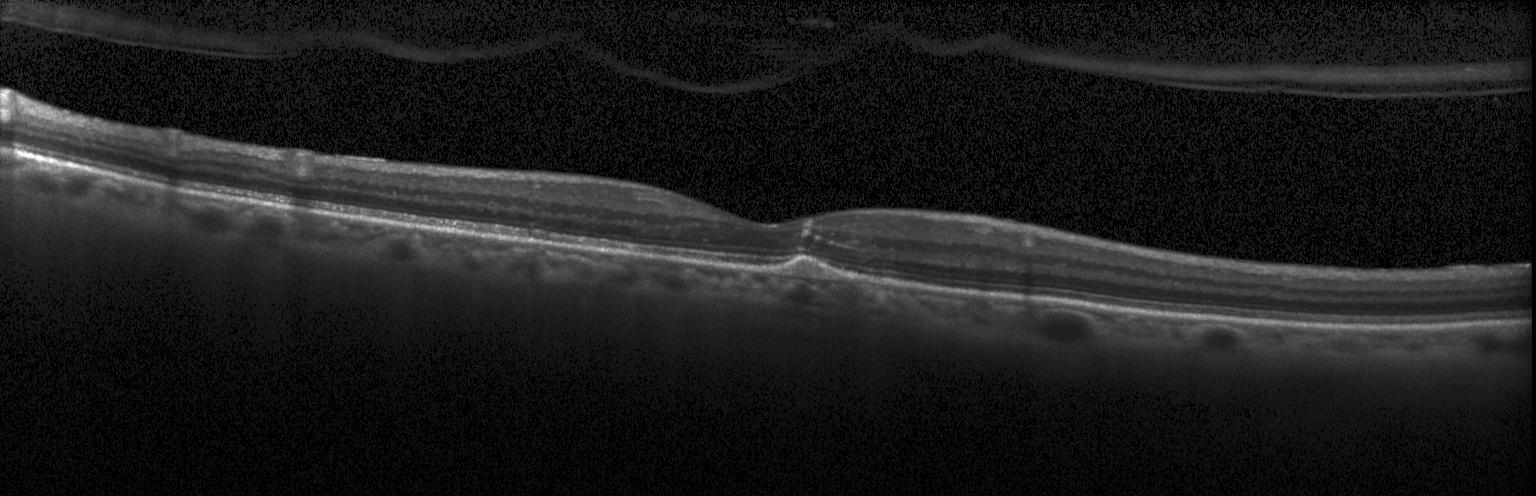
Spectral-domain OCT B-scan: a choroidal neovascular membrane.